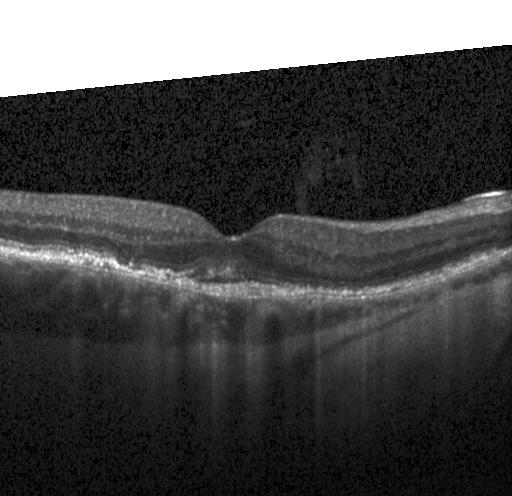 Instrument: Heidelberg Spectralis; OCT line scan; SD-OCT. The scan shows CNV.